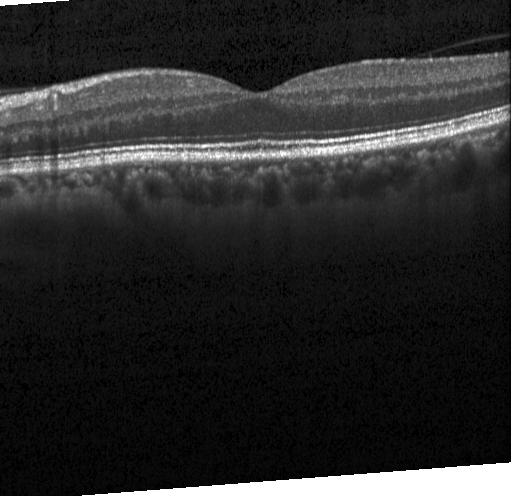 Heidelberg Spectralis OCT system, through the macula, retinal OCT B-scan, SD-OCT
No CNV, no DME, and no drusen.